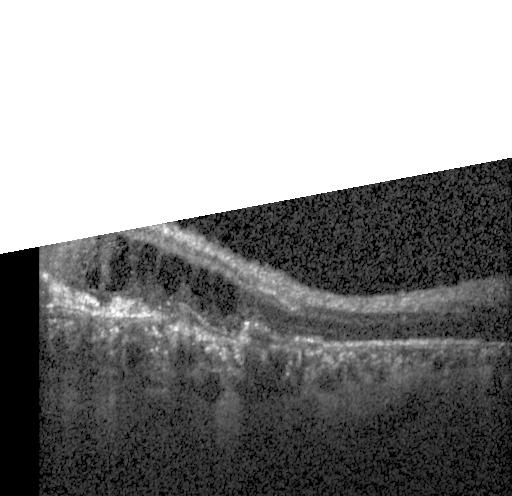 Optical coherence tomography scan. Horizontal scan through the fovea. Heidelberg Spectralis — Finding: choroidal neovascularization (CNV).